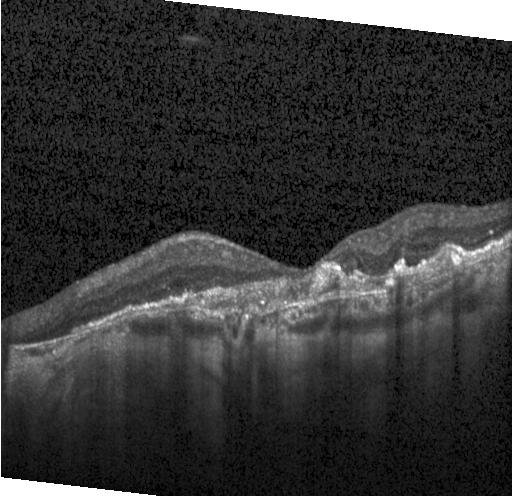 OCT B-scan · fovea-centered · acquired on a Heidelberg Spectralis. Dx: CNV.